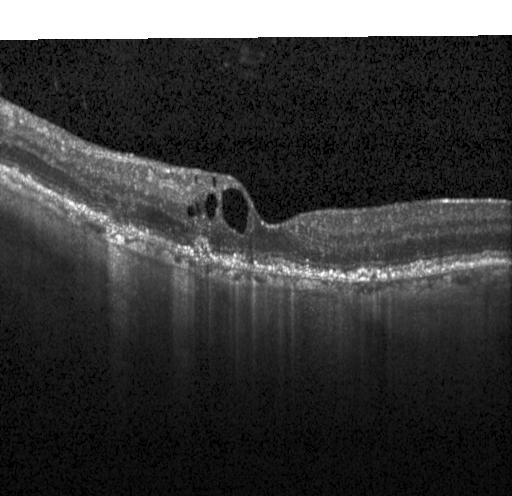

Impression: a choroidal neovascular membrane.